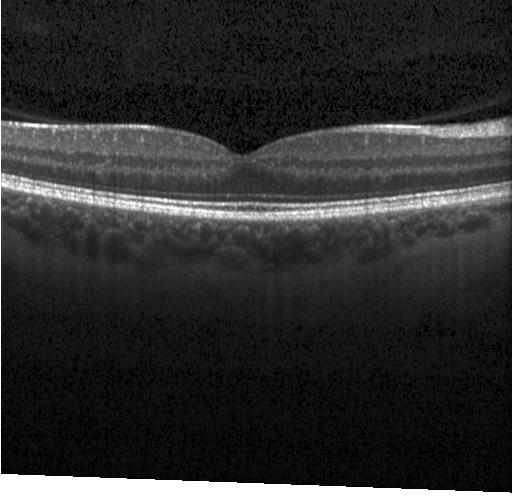

Retinal OCT B-scan · SD-OCT · fovea-centered.
Diagnosis: no CNV, no DME, and no drusen.